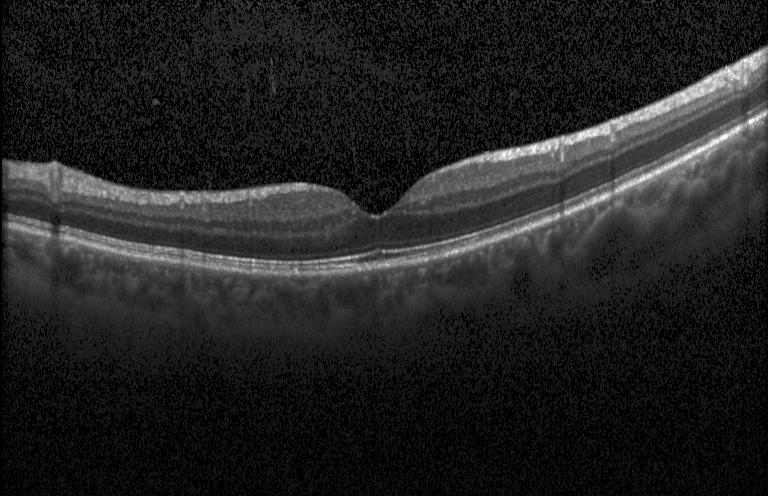
Macular scan · retinal OCT cross-section — Impression: no CNV, DME, or drusen.